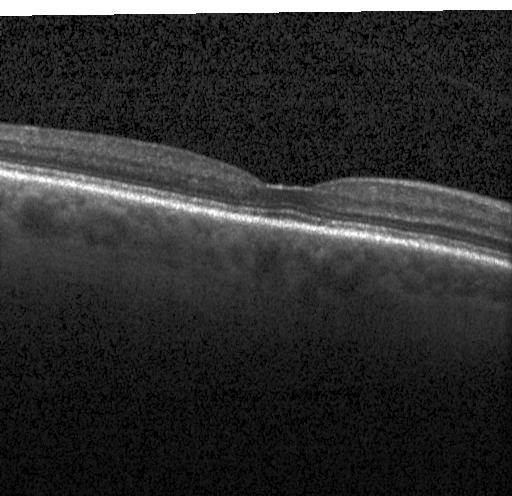
Retinal OCT cross-section.
Impression: no evidence of choroidal neovascularization, diabetic macular edema, or drusen.